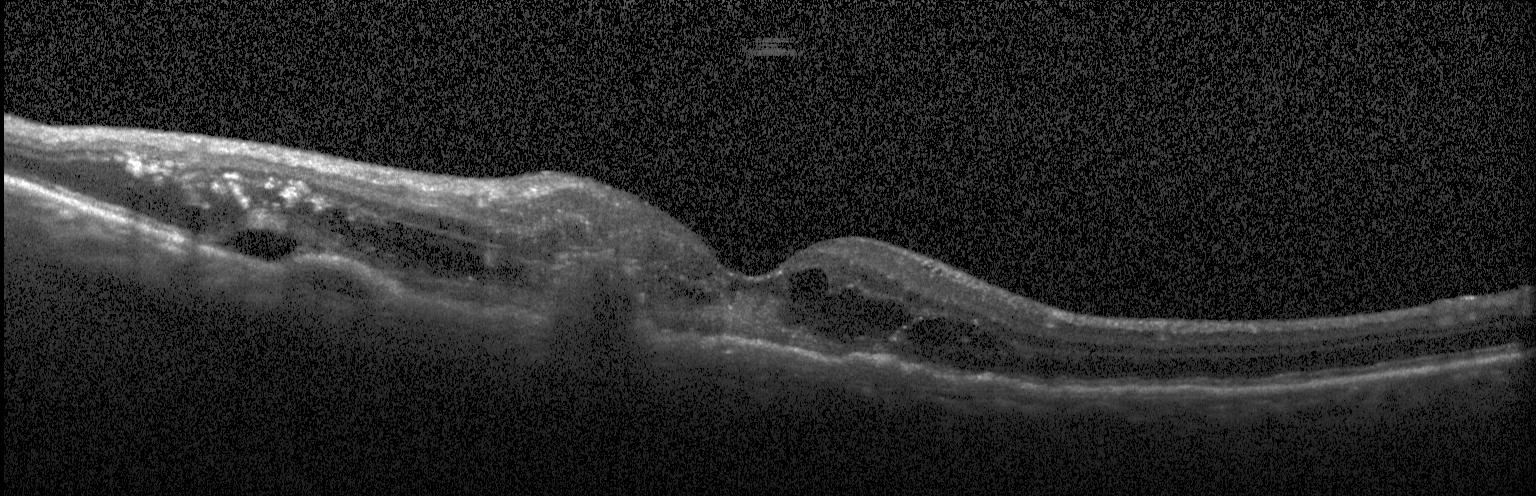
Retinal OCT cross-section. Spectral-domain optical coherence tomography. Instrument: Heidelberg Spectralis.
Diagnosis: choroidal neovascularization.